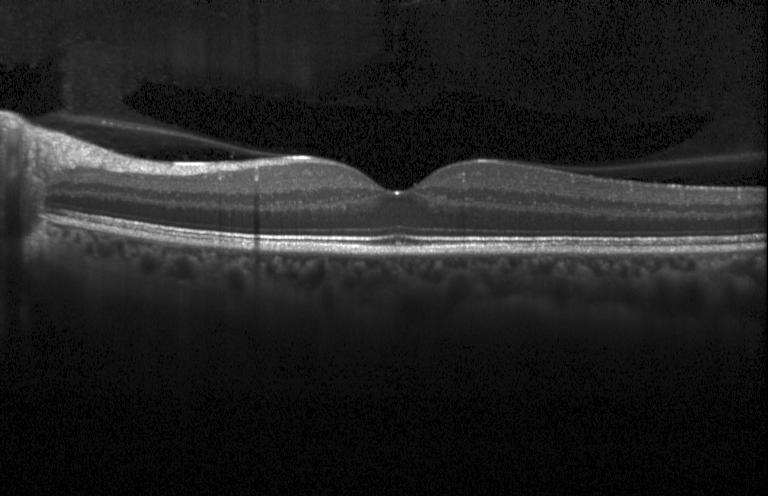
The scan shows no CNV, no DME, and no drusen.